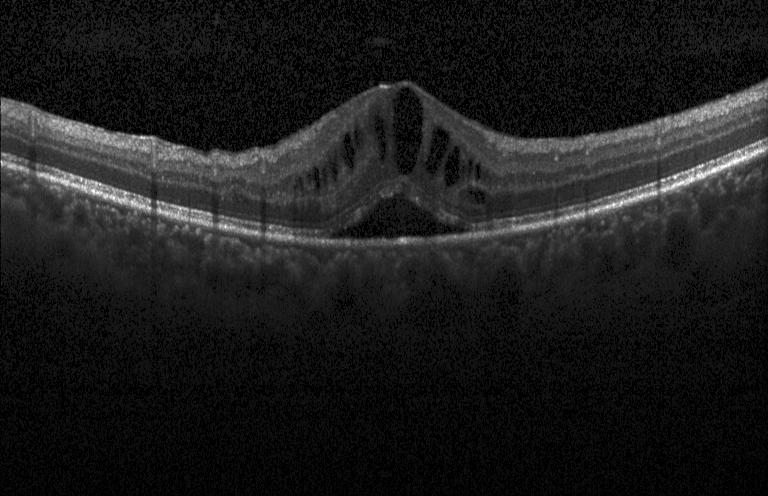 Macular OCT demonstrating diabetic macular edema.